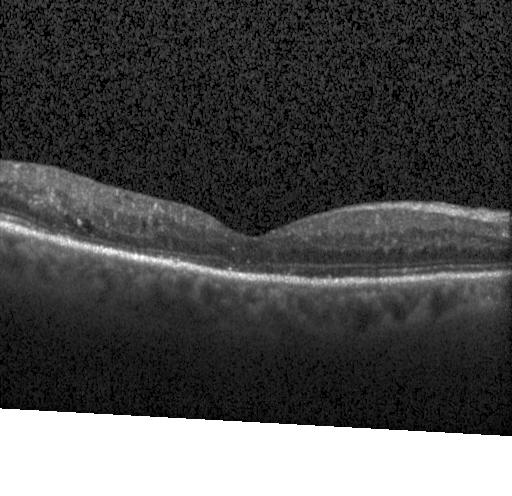

Macular scan. OCT B-scan — Impression: DME.